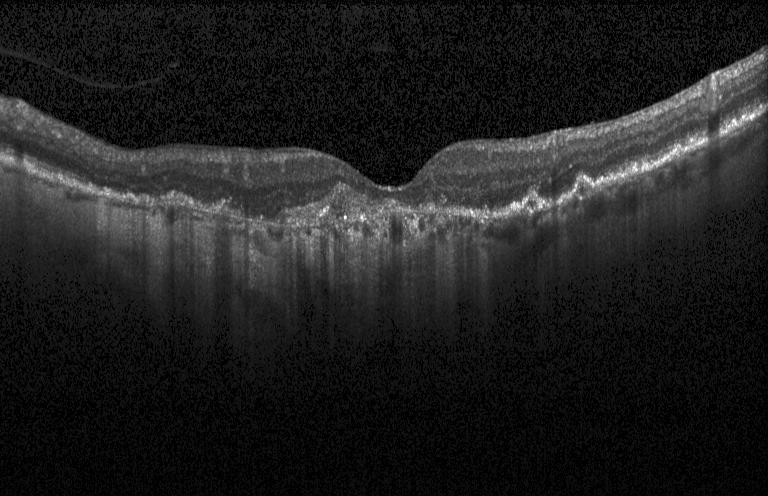 Macular scan · spectral-domain optical coherence tomography · optical coherence tomography B-scan · acquired on a Heidelberg Spectralis — The scan shows a choroidal neovascular membrane.